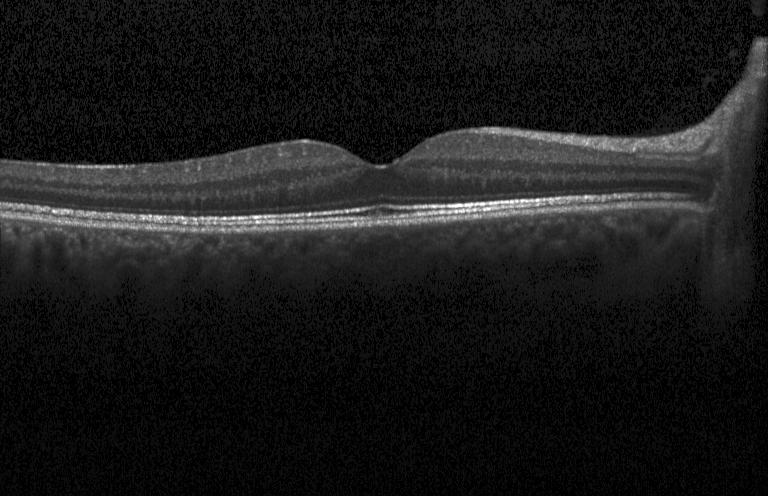
Impression: neither CNV, DME, nor drusen.